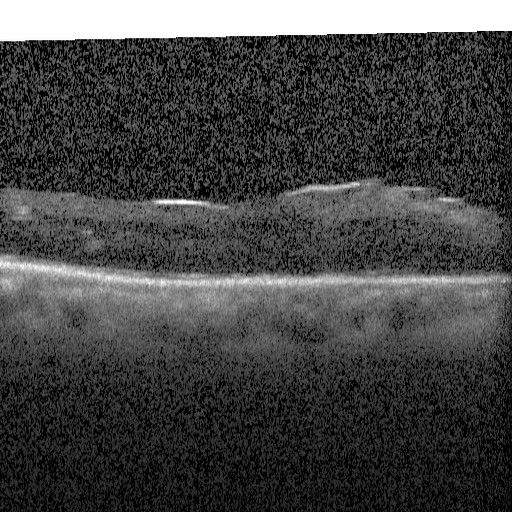 OCT line scan — Diagnosis: diabetic macular edema.